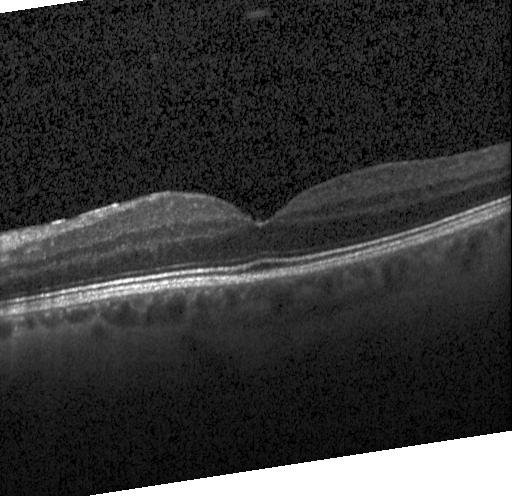
Diagnosis: no evidence of choroidal neovascularization, diabetic macular edema, or drusen.